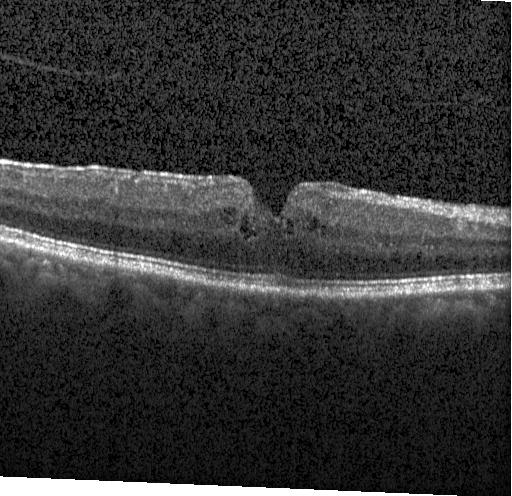
Acquired on a Heidelberg Spectralis; optical coherence tomography B-scan — Diabetic macular edema.